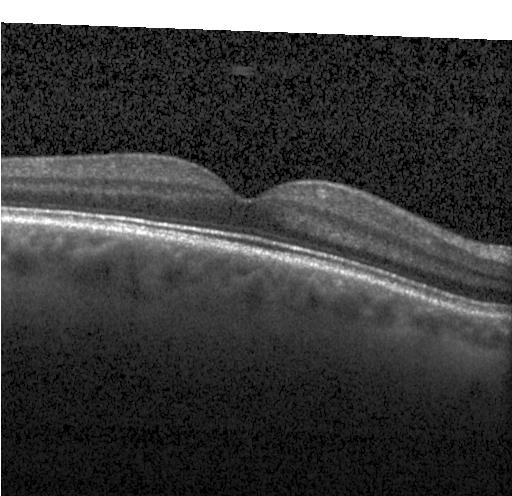

OCT finding: no evidence of CNV, DME, or drusen.